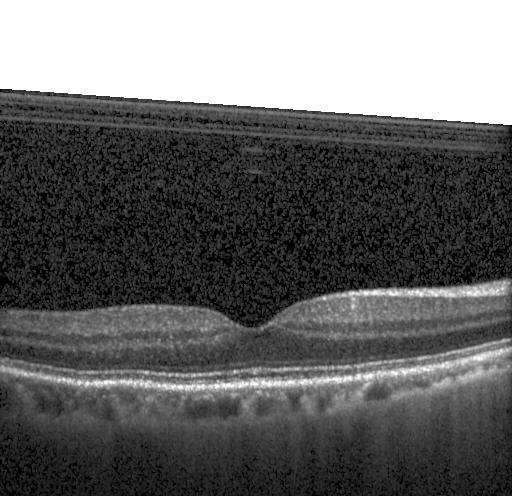
Impression: neither choroidal neovascularization, diabetic macular edema, nor drusen.